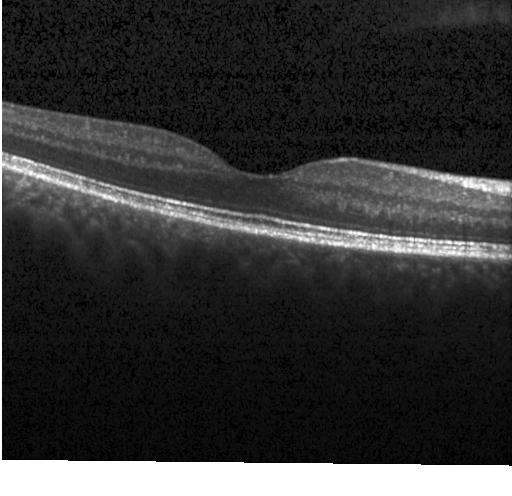
Impression: no evidence of choroidal neovascularization, diabetic macular edema, or drusen.